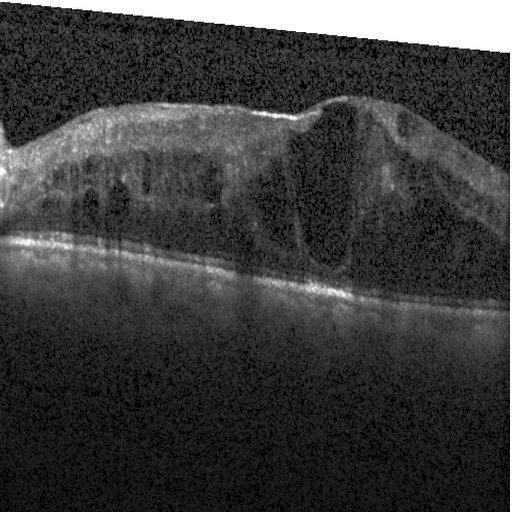
This B-scan demonstrates diabetic macular edema (DME).